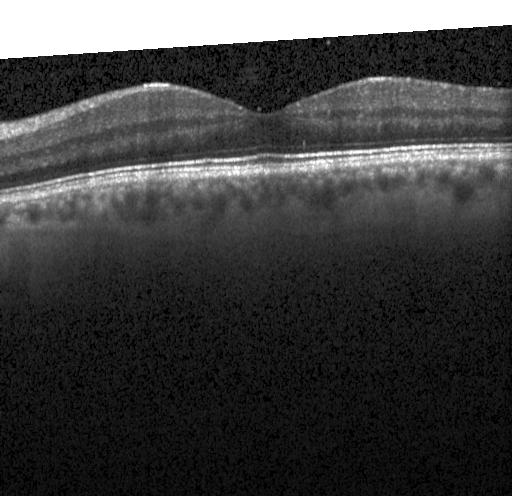

Retinal OCT cross-section; instrument: Heidelberg Spectralis; spectral-domain OCT. This B-scan demonstrates no choroidal neovascularization, diabetic macular edema, or drusen.